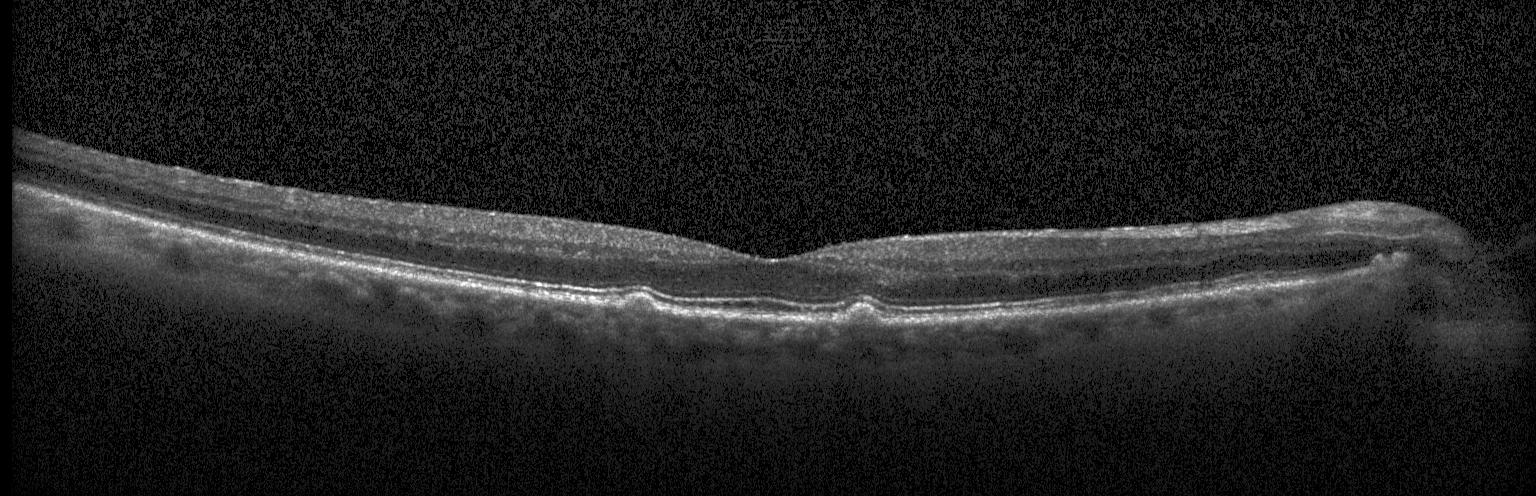
Macular scan; SD-OCT; OCT line scan; instrument: Heidelberg Spectralis — Diagnosis: drusen.